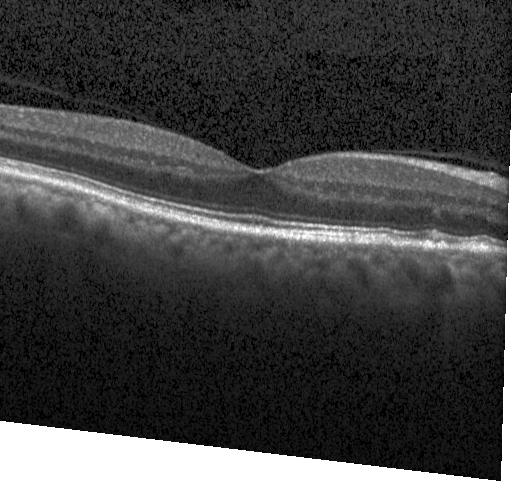 Macular OCT demonstrating drusen.